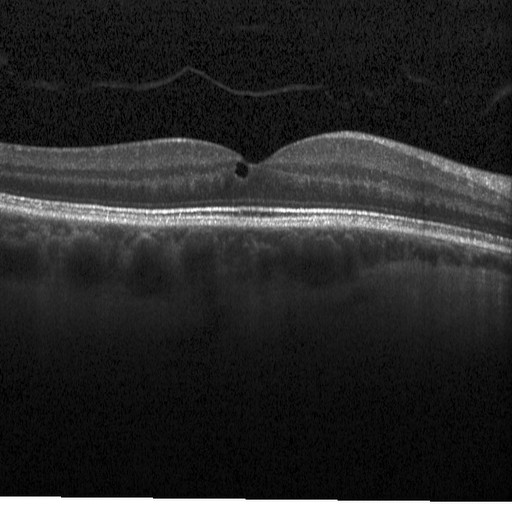
Retinal OCT B-scan, centered on the fovea, Heidelberg Spectralis OCT system. Impression: diabetic macular edema (DME).